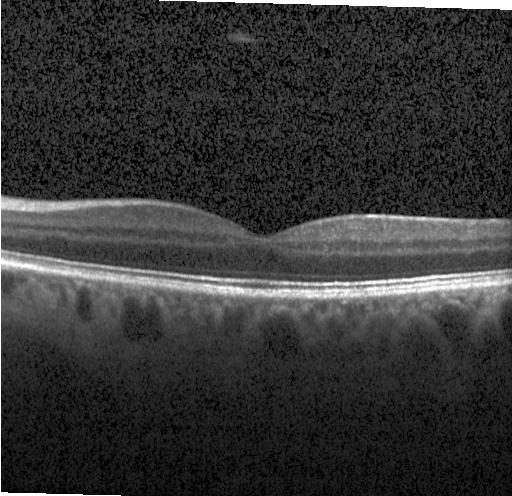
Retinal OCT cross-section showing no choroidal neovascularization, diabetic macular edema, or drusen.